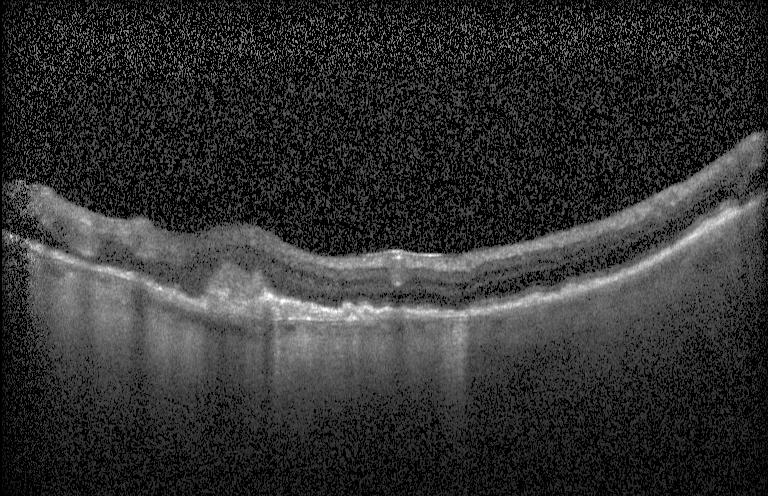

Spectral-domain OCT B-scan: choroidal neovascularization (CNV).